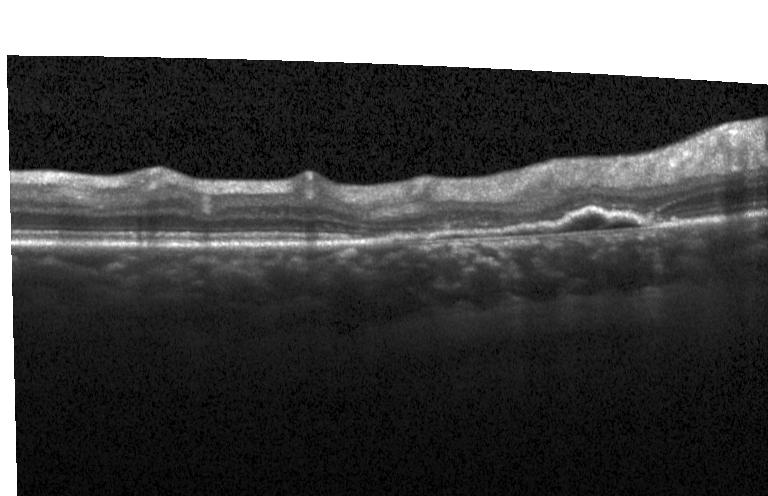

Centered on the fovea; retinal OCT cross-section. OCT finding: CNV.